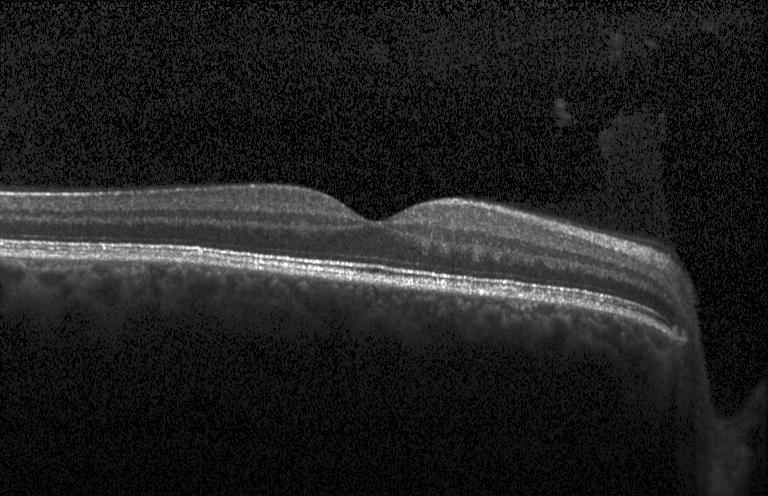
This B-scan demonstrates no choroidal neovascularization, diabetic macular edema, or drusen.